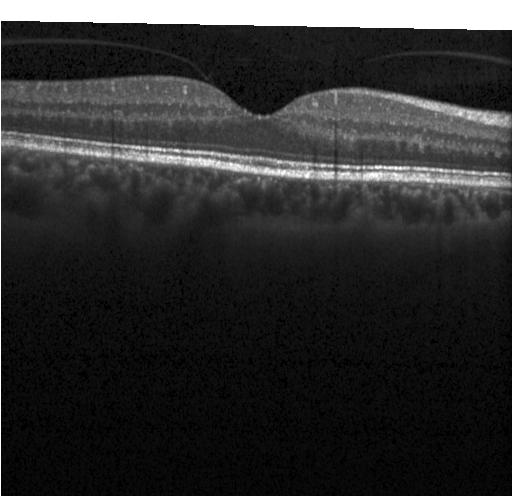 Horizontal scan through the fovea · retinal OCT cross-section · SD-OCT. Impression: no evidence of choroidal neovascularization, diabetic macular edema, or drusen.